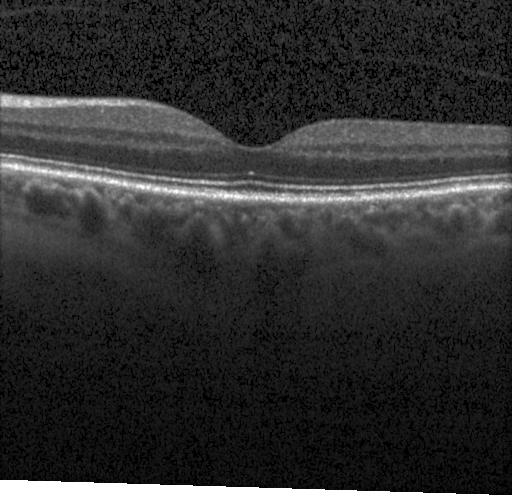
OCT B-scan; acquired on a Heidelberg Spectralis. Diagnosis: neither CNV, DME, nor drusen.